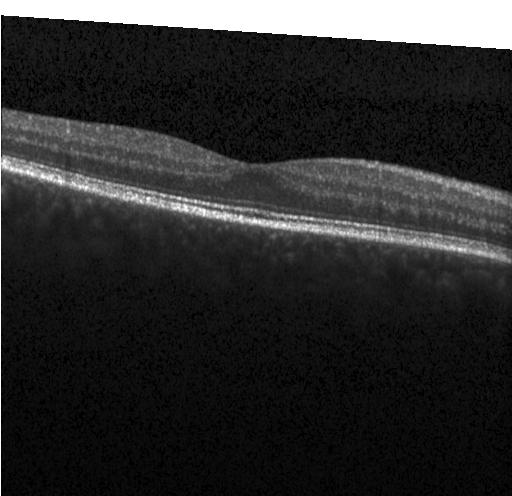

Retinal OCT B-scan — This B-scan demonstrates neither CNV, DME, nor drusen.